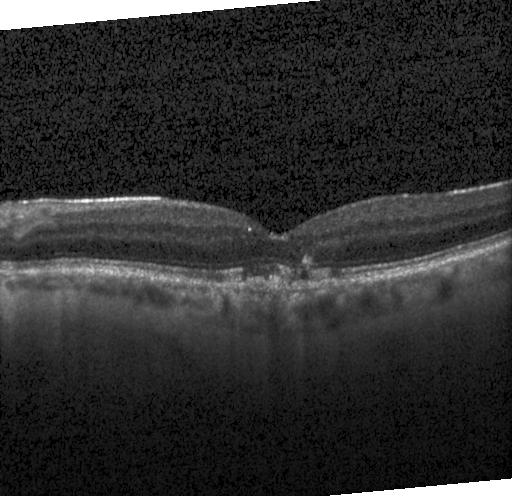
OCT B-scan showing a choroidal neovascular membrane.